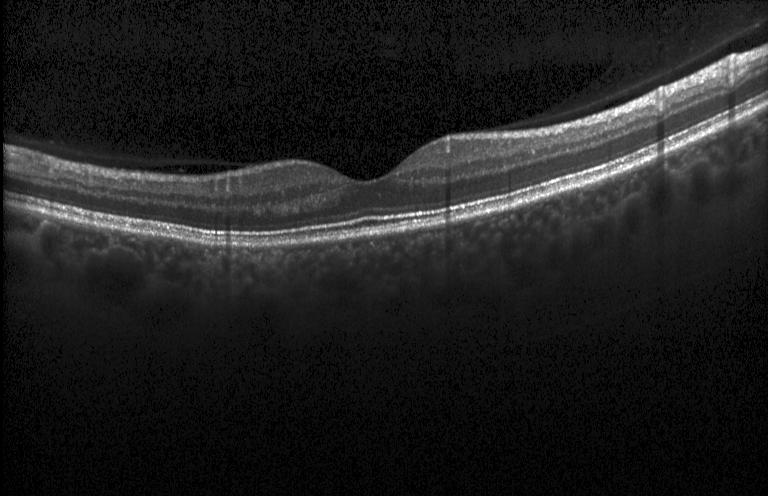
Impression: no choroidal neovascularization, diabetic macular edema, or drusen.